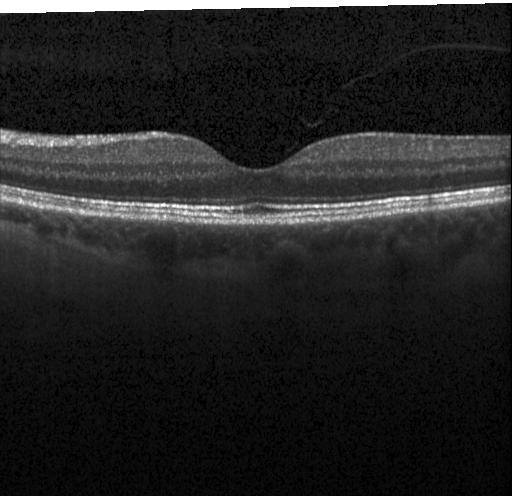

Diagnosis: neither choroidal neovascularization, diabetic macular edema, nor drusen.